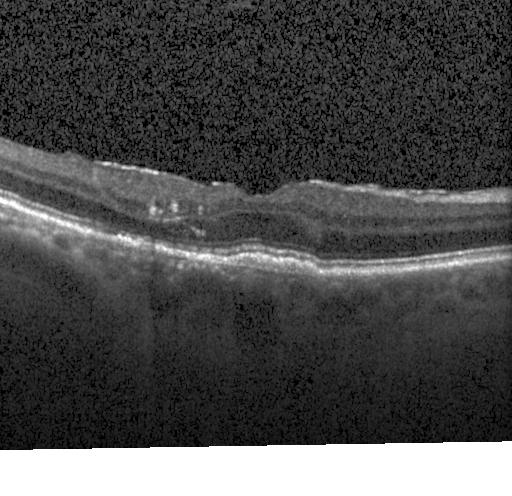
Impression: a choroidal neovascular membrane.